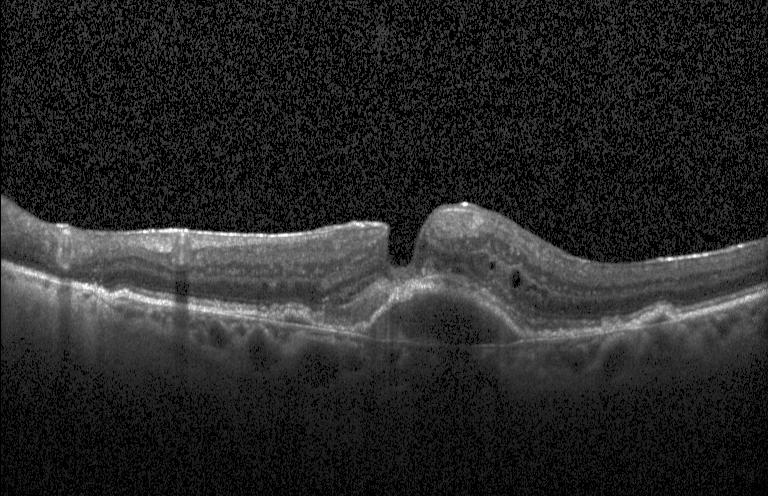 Spectral-domain optical coherence tomography; horizontal scan through the fovea; Heidelberg Spectralis; optical coherence tomography scan — Impression: a choroidal neovascular membrane.